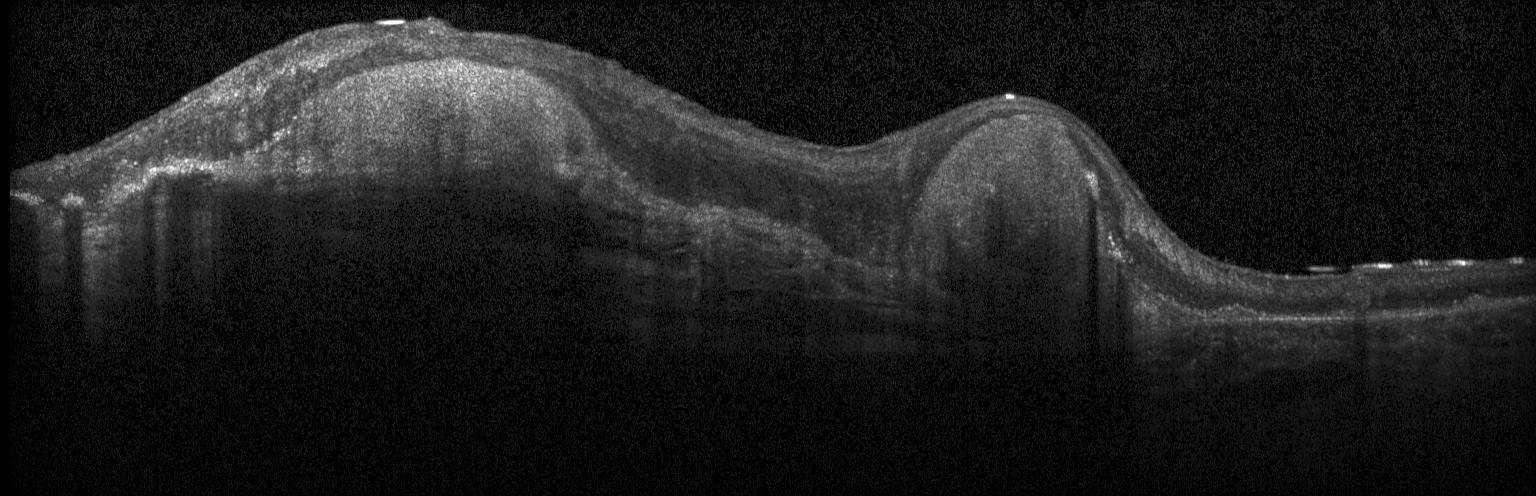
Macular OCT demonstrating CNV.